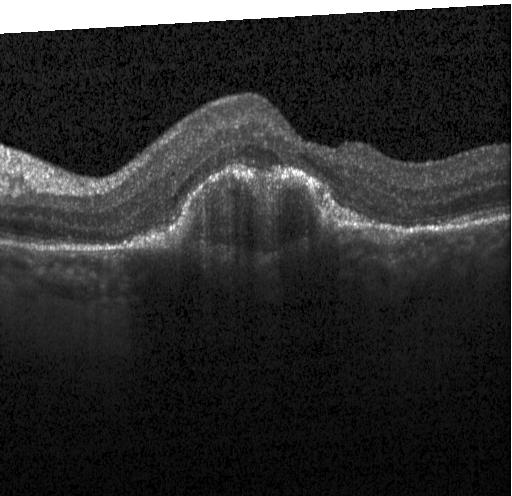

Spectral-domain optical coherence tomography. OCT B-scan. Heidelberg Spectralis
Macular OCT: a choroidal neovascular membrane.